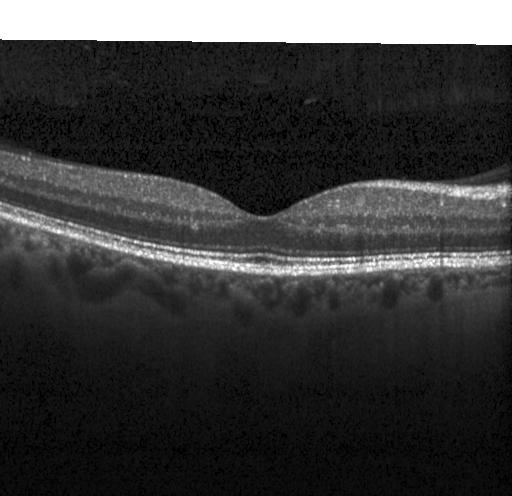
Optical coherence tomography B-scan — Impression: no evidence of CNV, DME, or drusen.